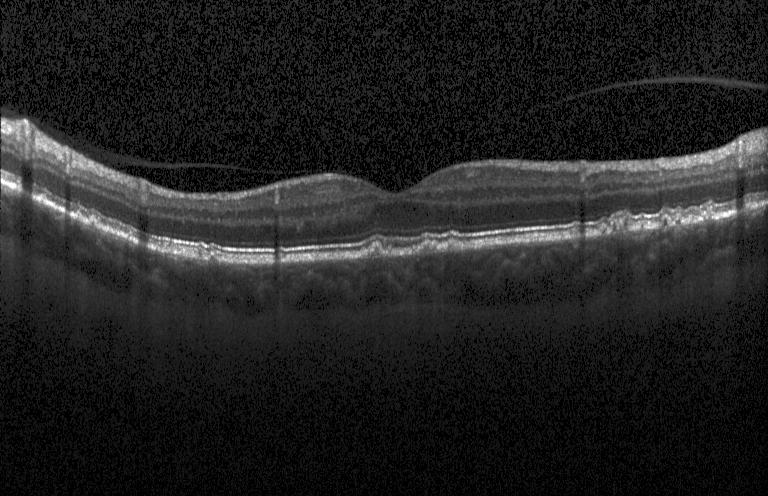 Spectral-domain optical coherence tomography. Through the macula. Retinal OCT B-scan. Instrument: Heidelberg Spectralis
Sub-RPE drusenoid deposits.